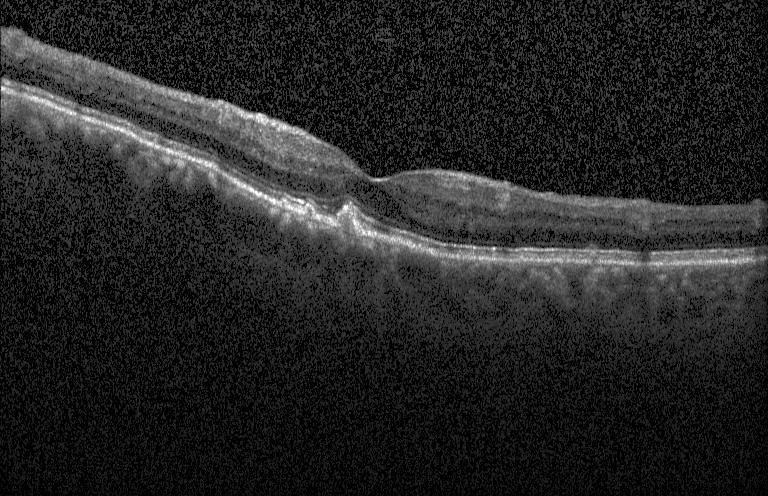

Impression: multiple drusen.